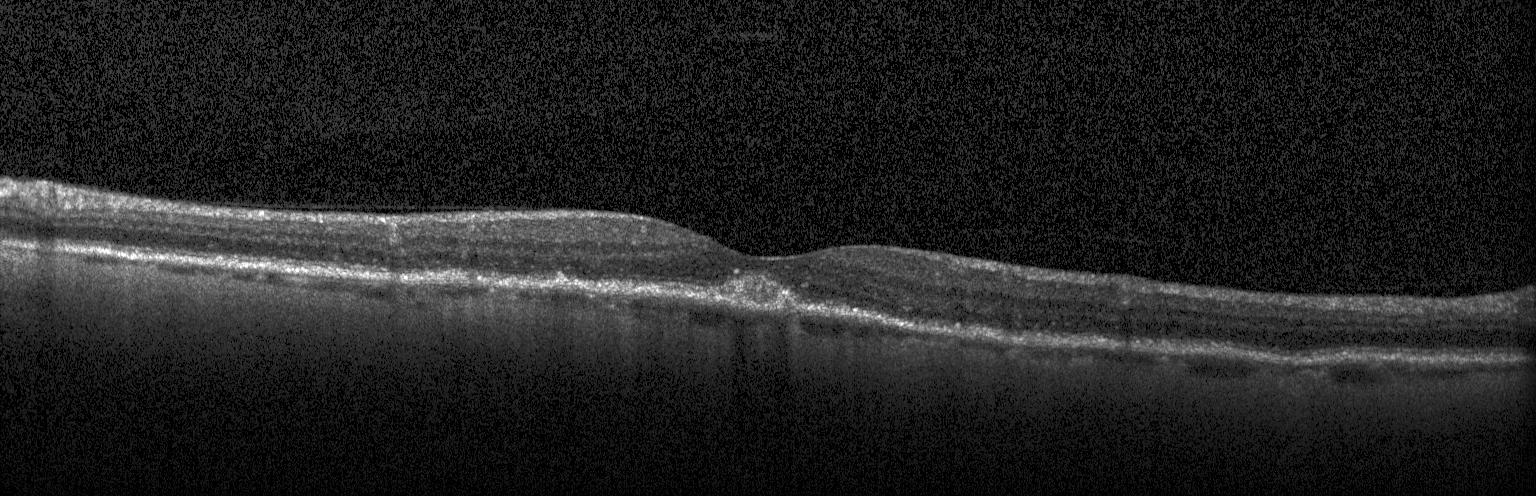
Heidelberg Spectralis · optical coherence tomography scan · macular scan · spectral-domain optical coherence tomography.
Impression: sub-RPE drusenoid deposits.